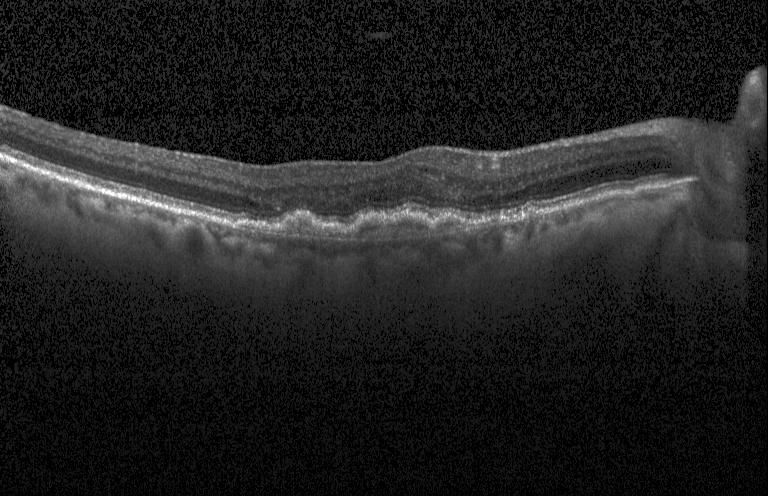 OCT B-scan. SD-OCT. Through the macula.
OCT finding: a choroidal neovascular membrane.